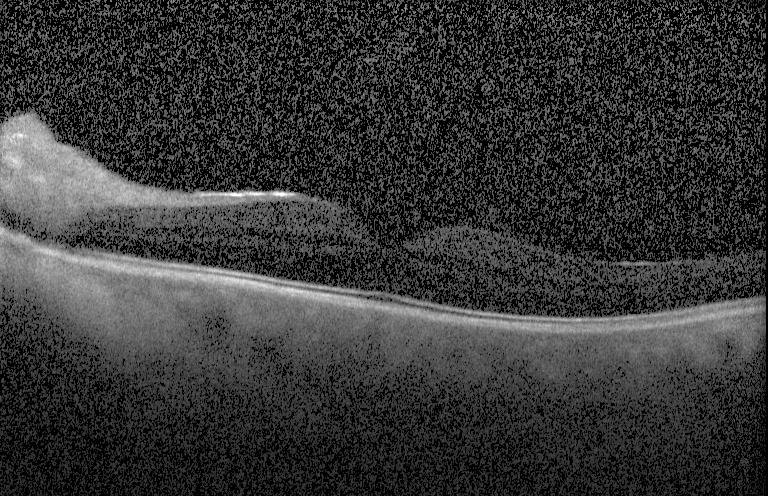
No evidence of CNV, DME, or drusen.